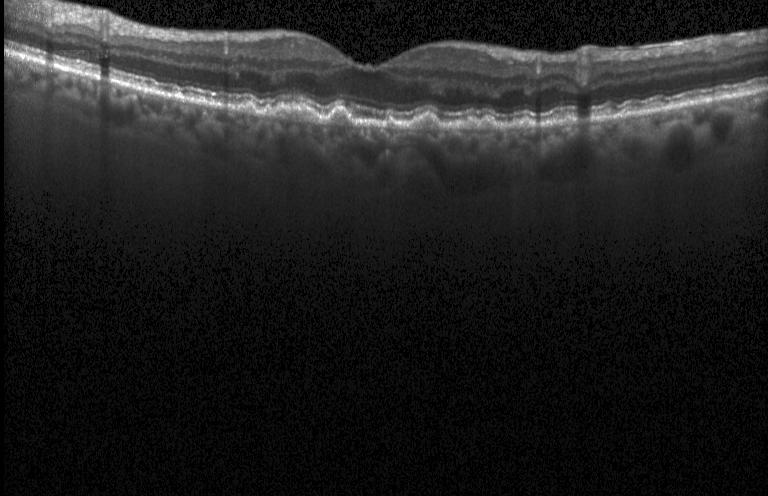
Drusen.